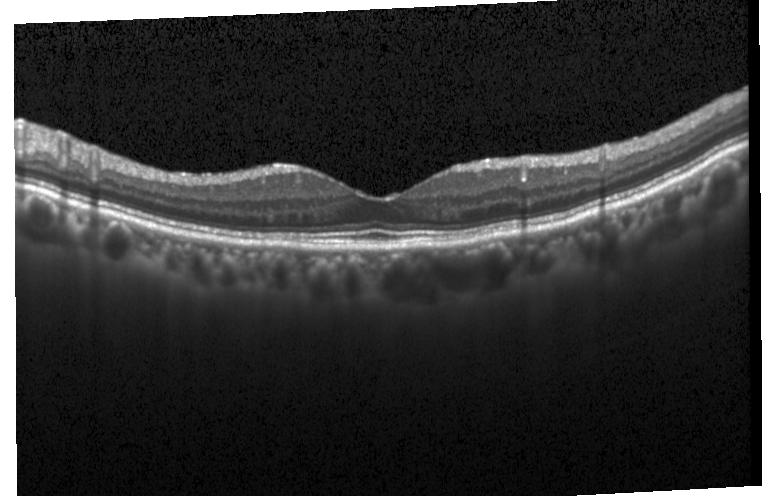 Spectral-domain OCT B-scan: no evidence of CNV, DME, or drusen.